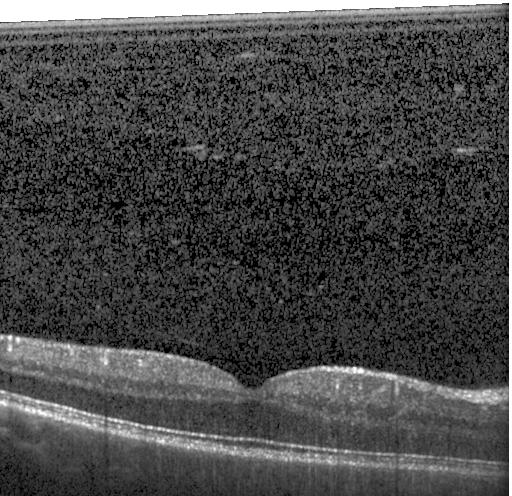 The scan shows no choroidal neovascularization, no diabetic macular edema, and no drusen.